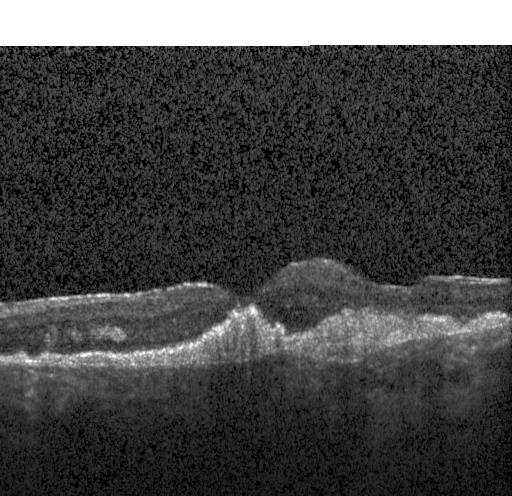
This B-scan demonstrates a choroidal neovascular membrane.